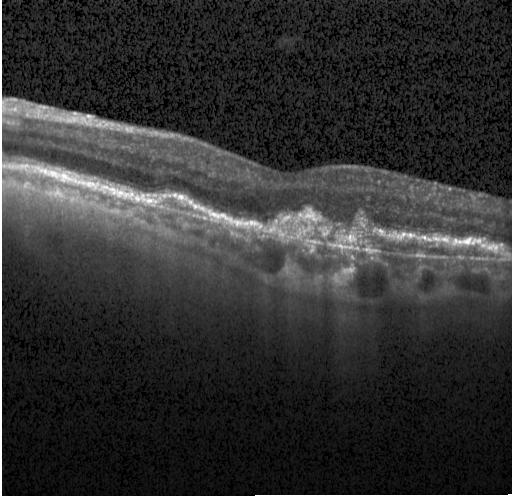

Finding: choroidal neovascularization (CNV).